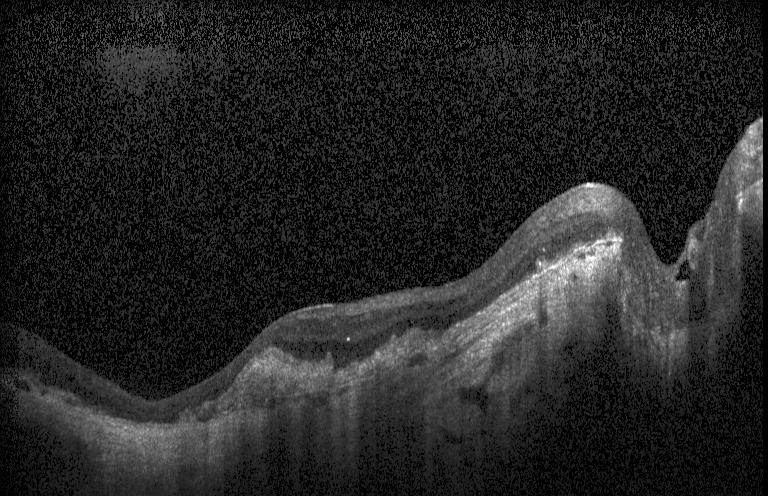 OCT B-scan showing choroidal neovascularization (CNV).